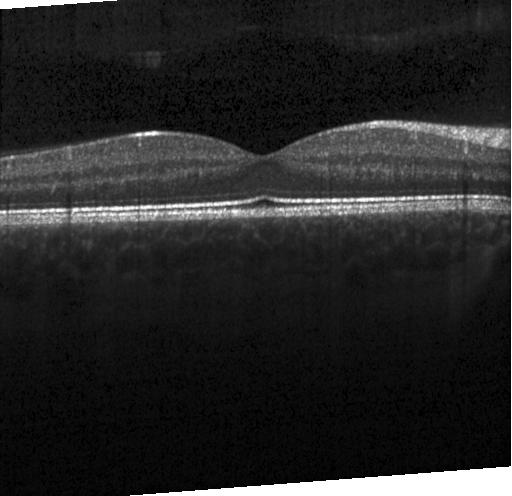
The scan shows no CNV, DME, or drusen.